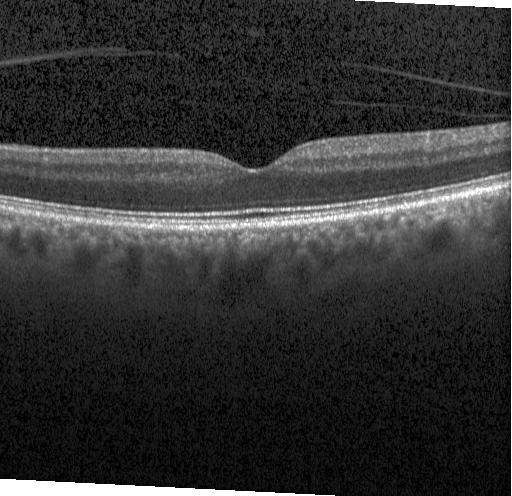

Spectral-domain OCT, retinal OCT B-scan, horizontal scan through the fovea, Heidelberg Spectralis OCT system
Diagnosis: no choroidal neovascularization, no diabetic macular edema, and no drusen.